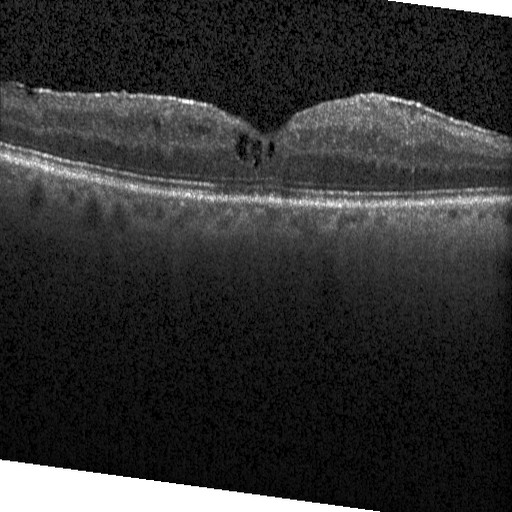

Retinal OCT cross-section — Macular OCT: DME.